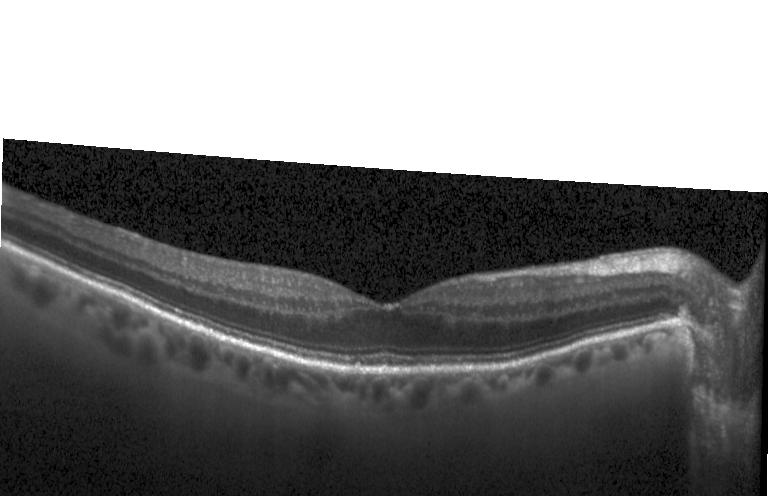

OCT line scan.
Neither choroidal neovascularization, diabetic macular edema, nor drusen.